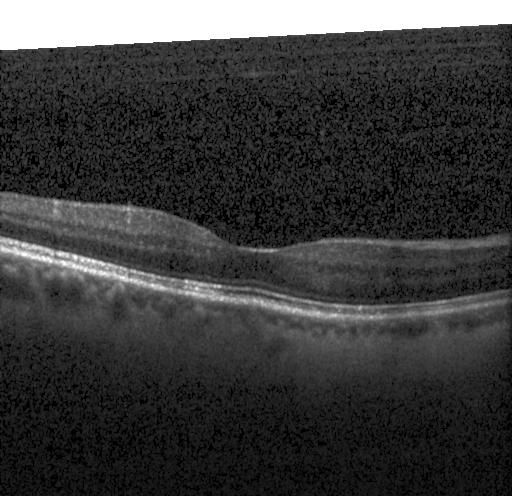
SD-OCT; acquired on a Heidelberg Spectralis; retinal OCT cross-section; horizontal scan through the fovea. Diagnosis: no evidence of choroidal neovascularization, diabetic macular edema, or drusen.